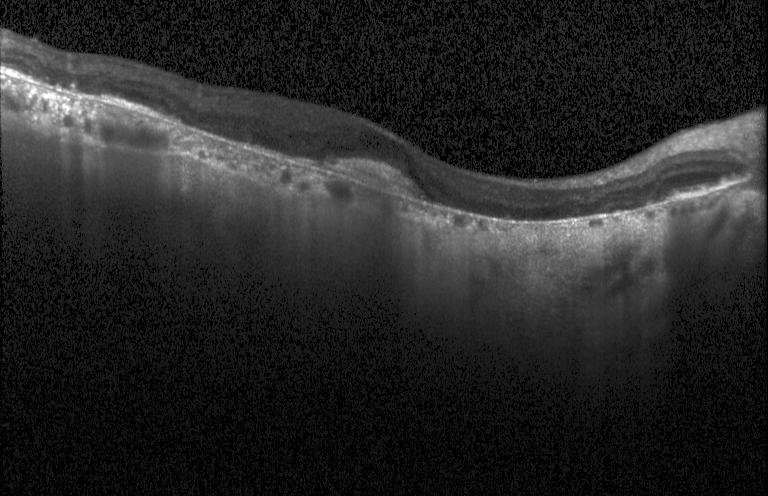

Macular OCT: choroidal neovascularization (CNV).